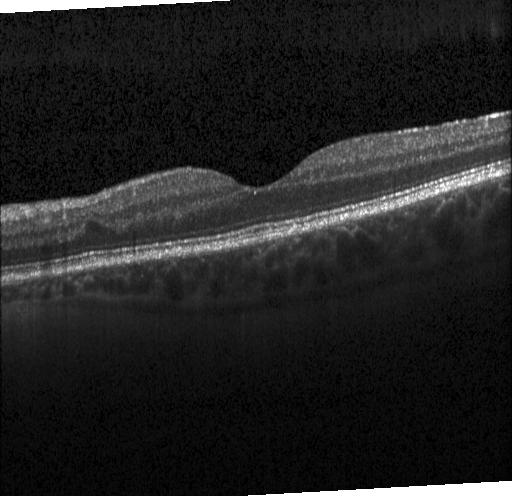

Impression: no evidence of choroidal neovascularization, diabetic macular edema, or drusen.